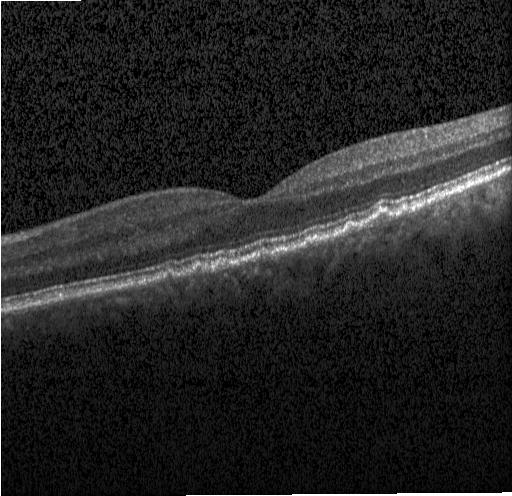
Optical coherence tomography scan. Acquired on a Heidelberg Spectralis.
Assessment: sub-RPE drusenoid deposits.